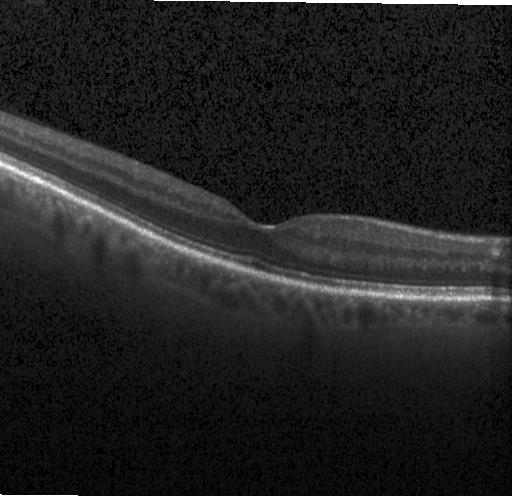 Assessment: neither choroidal neovascularization, diabetic macular edema, nor drusen.